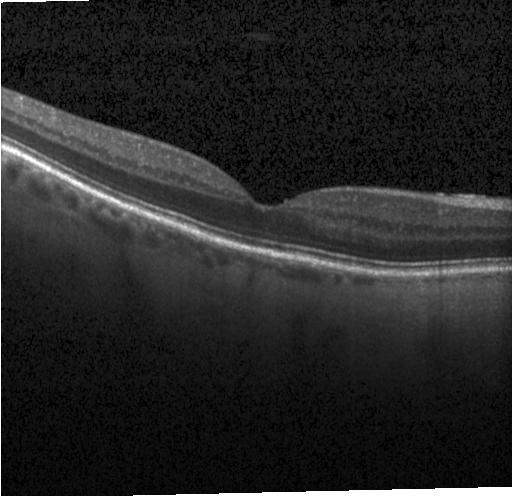

SD-OCT · horizontal scan through the fovea · optical coherence tomography scan · acquired on a Heidelberg Spectralis
The scan shows no choroidal neovascularization, diabetic macular edema, or drusen.